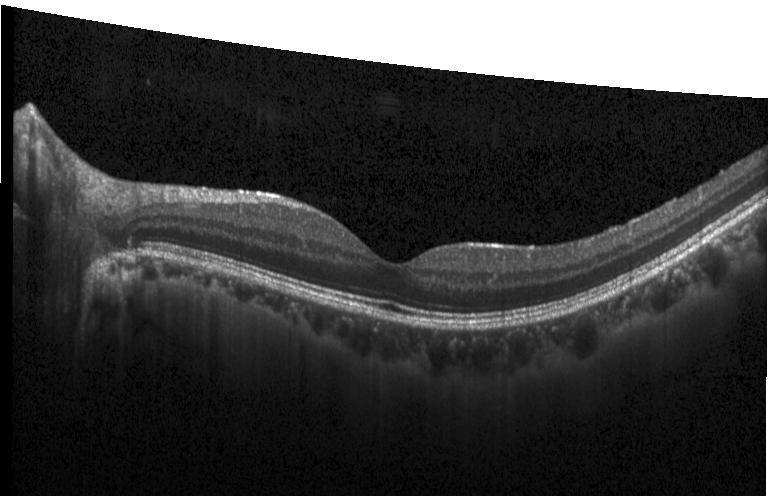

Finding: no evidence of choroidal neovascularization, diabetic macular edema, or drusen.